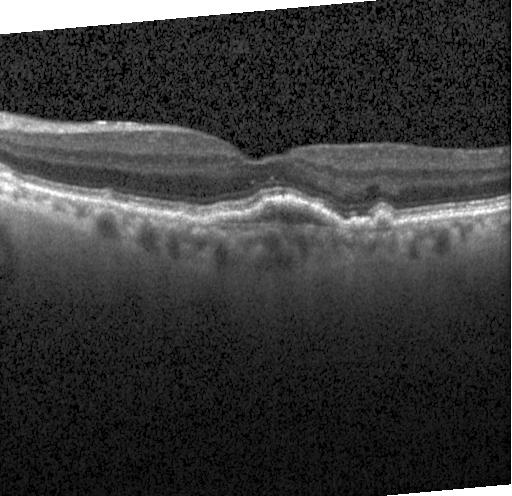 Diagnosis: choroidal neovascularization (CNV).